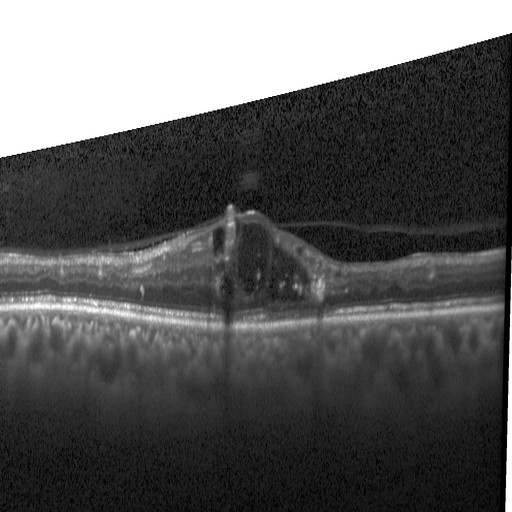 Spectral-domain OCT B-scan: diabetic macular edema.